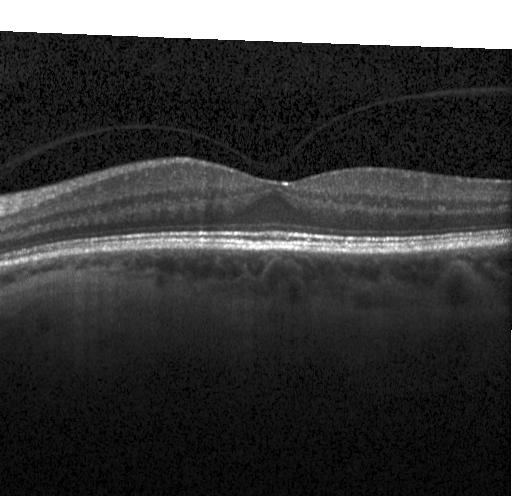
Spectral-domain optical coherence tomography. Horizontal scan through the fovea. Optical coherence tomography scan
Macular OCT: no evidence of choroidal neovascularization, diabetic macular edema, or drusen.